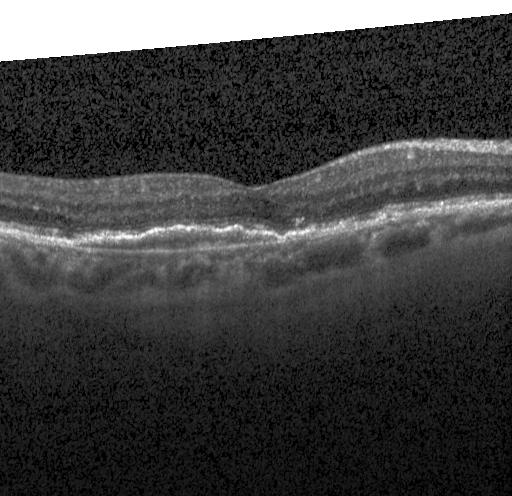

OCT B-scan · spectral-domain OCT · centered on the fovea. Assessment: CNV.